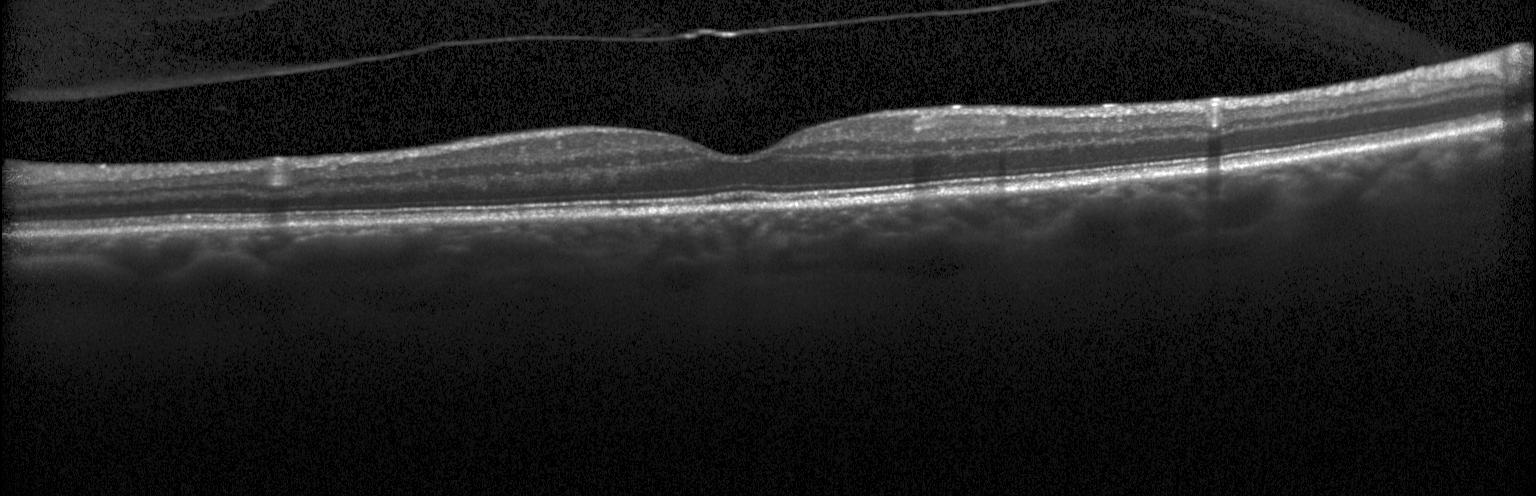
Acquired on a Heidelberg Spectralis. Macular scan. Optical coherence tomography B-scan. Spectral-domain OCT.
Diagnosis: no evidence of choroidal neovascularization, diabetic macular edema, or drusen.